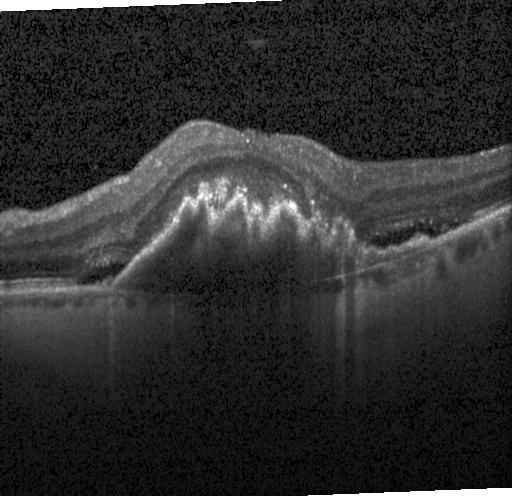 OCT finding: a choroidal neovascular membrane.